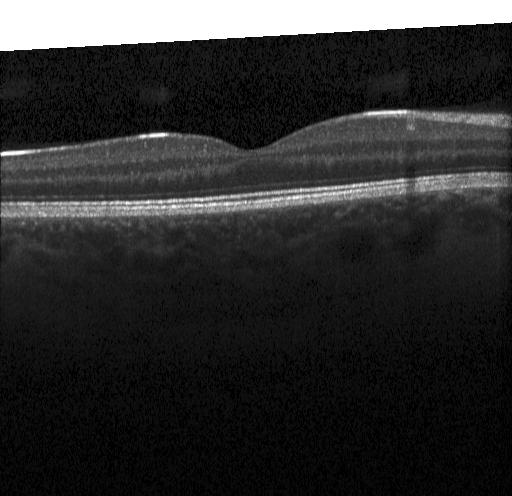 Retinal OCT B-scan · through the macula · acquired on a Heidelberg Spectralis.
No evidence of choroidal neovascularization, diabetic macular edema, or drusen.